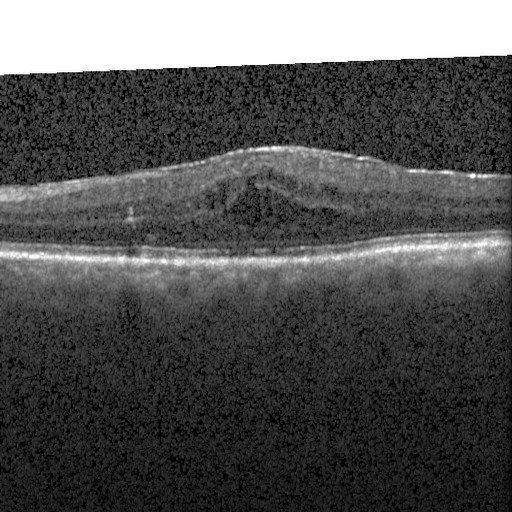

Finding: diabetic macular edema (DME).